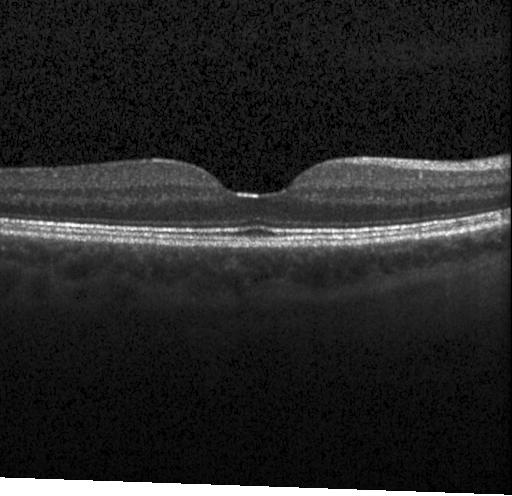

Impression: no choroidal neovascularization, diabetic macular edema, or drusen.